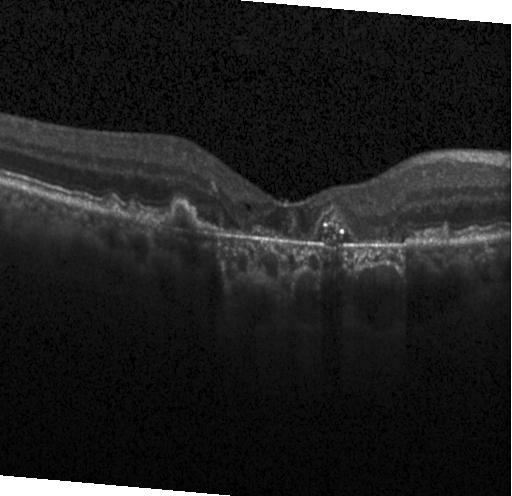 Dx: a choroidal neovascular membrane.